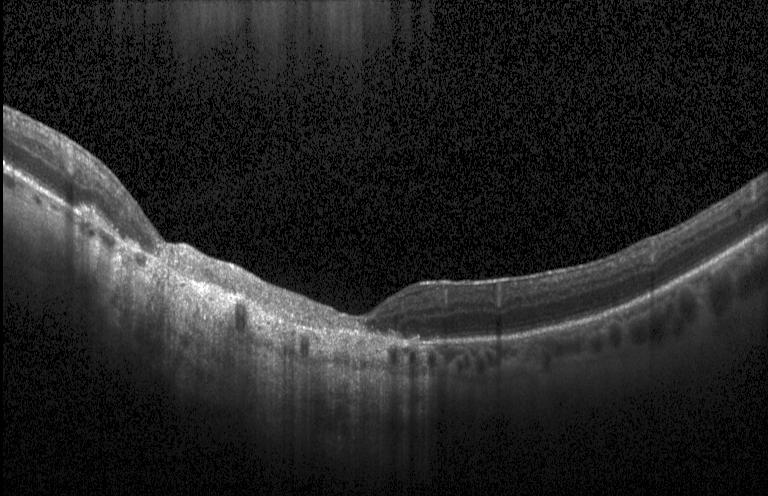

Optical coherence tomography scan.
Dx: a choroidal neovascular membrane.